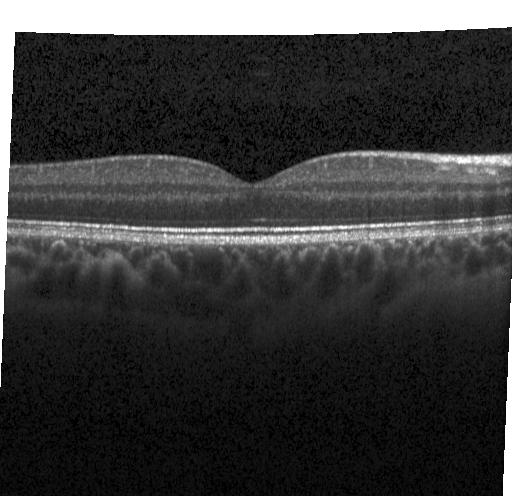

Fovea-centered. SD-OCT. Instrument: Heidelberg Spectralis. Retinal OCT B-scan
Impression: neither CNV, DME, nor drusen.